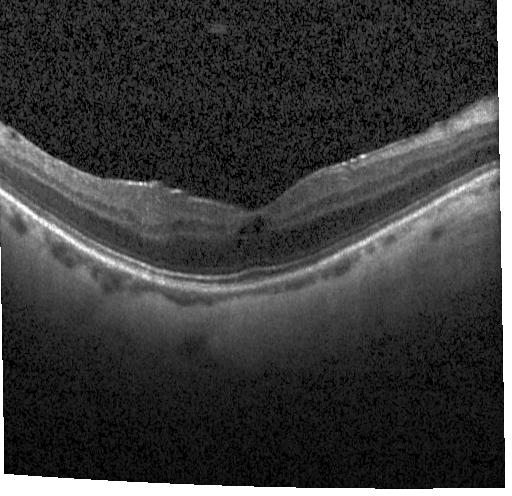

Diagnosis: diabetic macular edema (DME).